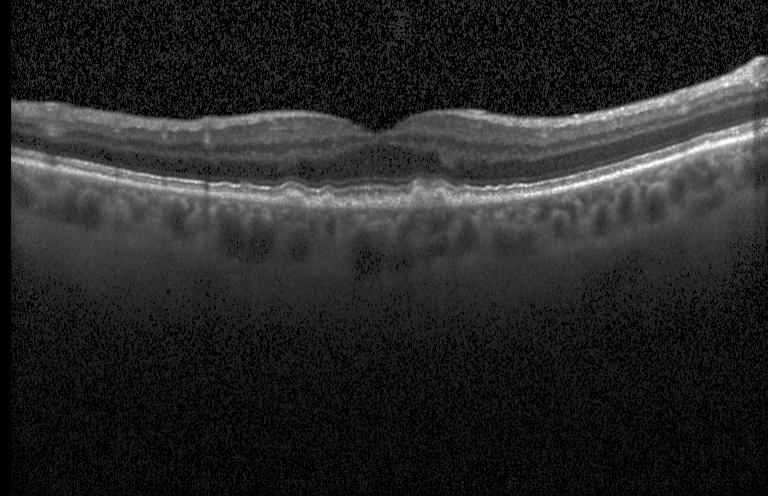
Multiple drusen.